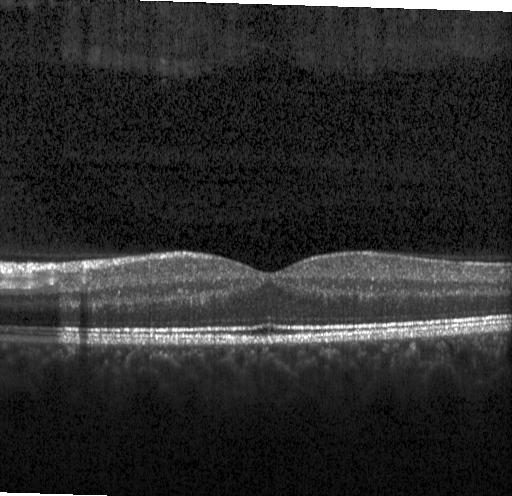 Macular OCT: no evidence of choroidal neovascularization, diabetic macular edema, or drusen.